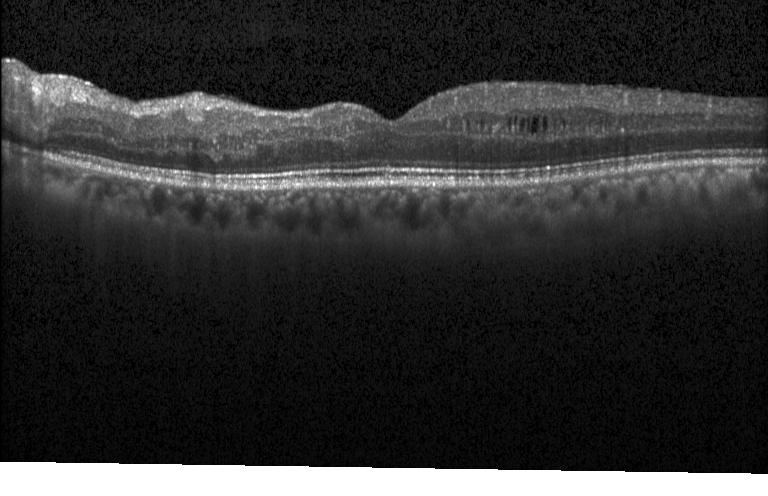
Optical coherence tomography scan, horizontal scan through the fovea, spectral-domain OCT, instrument: Heidelberg Spectralis
This B-scan demonstrates DME.